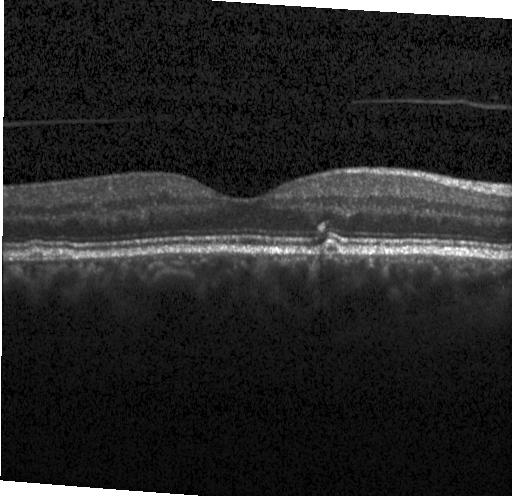

Through the macula. Optical coherence tomography B-scan
OCT finding: multiple drusen.